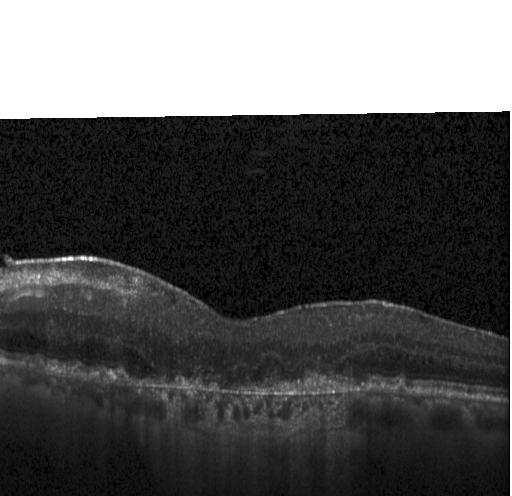 Retinal OCT B-scan · macular scan
Diagnosis: a choroidal neovascular membrane.